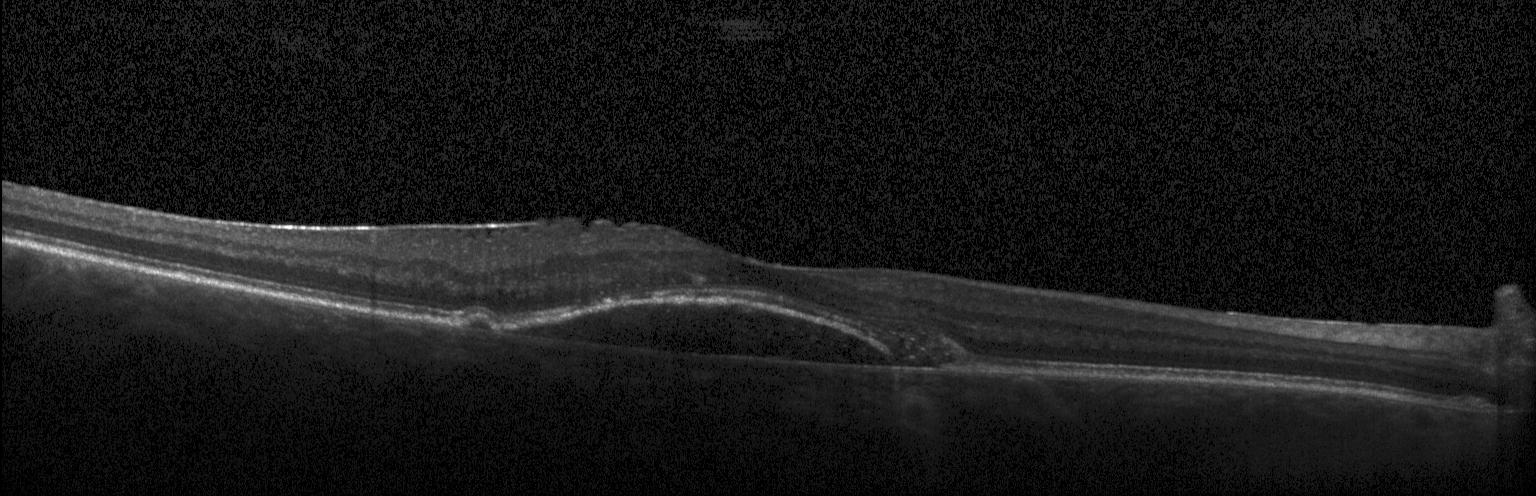

Optical coherence tomography B-scan.
Dx: CNV.